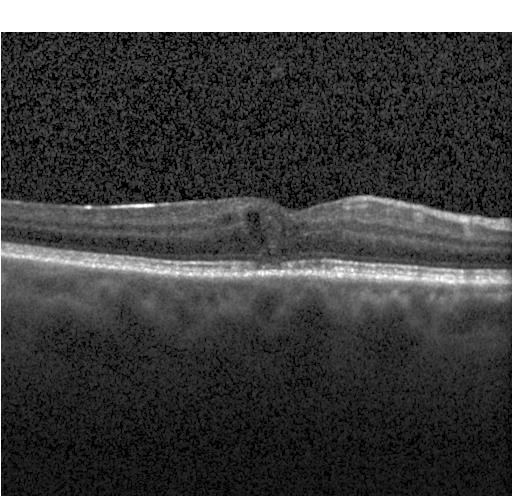
OCT line scan
DME.